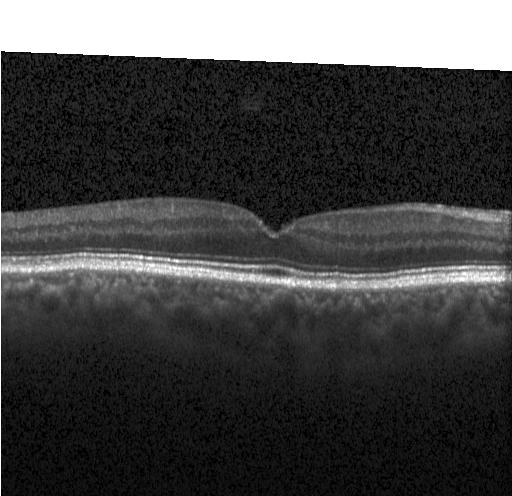

Impression: no CNV, no DME, and no drusen.